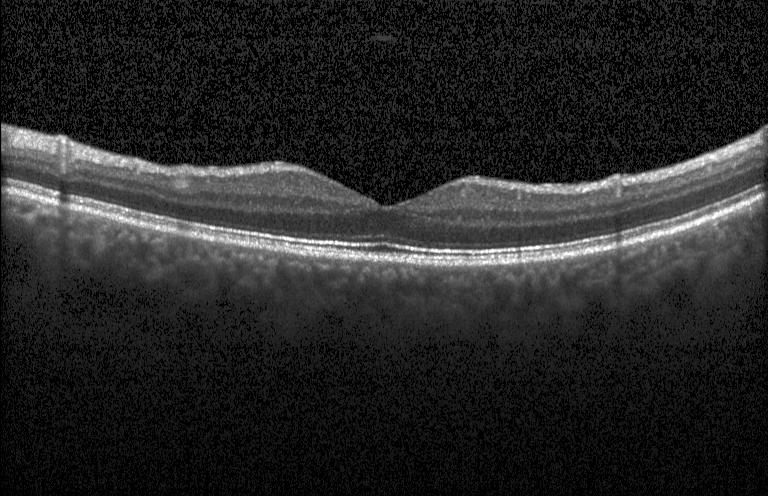
Impression: no CNV, no DME, and no drusen.